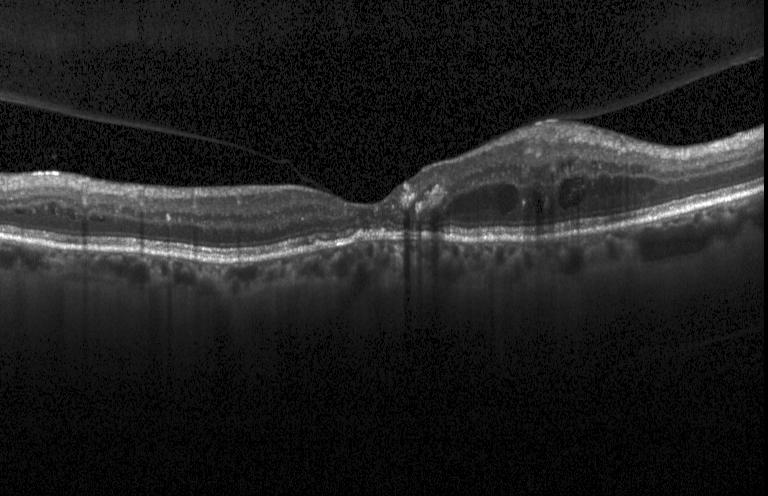

Centered on the fovea. Instrument: Heidelberg Spectralis. OCT line scan. SD-OCT.
Impression: a choroidal neovascular membrane.